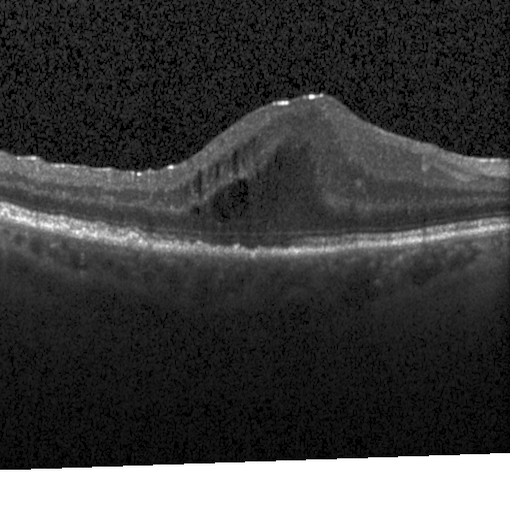 Heidelberg Spectralis; spectral-domain optical coherence tomography; through the macula; retinal OCT cross-section — This B-scan demonstrates DME.